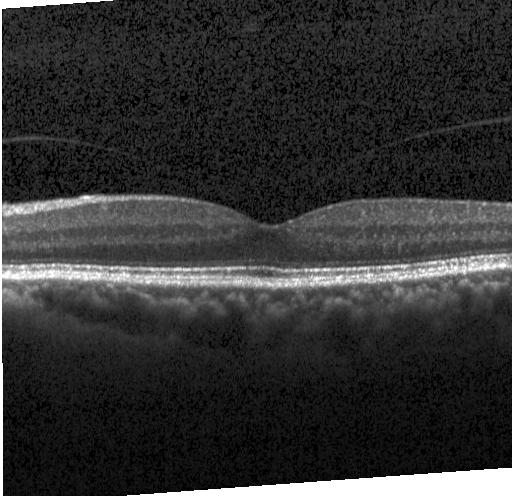

Diagnosis: neither choroidal neovascularization, diabetic macular edema, nor drusen.